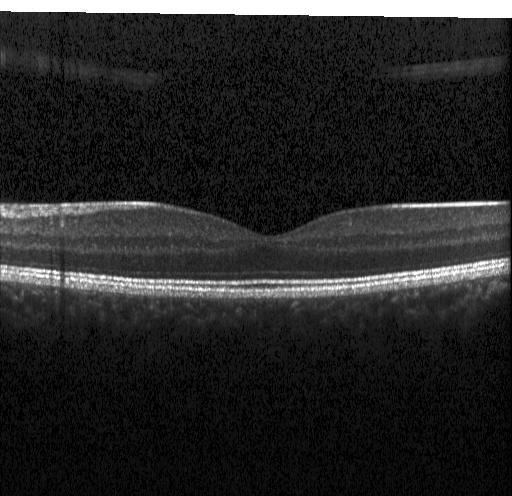 Fovea-centered; retinal OCT cross-section
Diagnosis: no choroidal neovascularization, no diabetic macular edema, and no drusen.